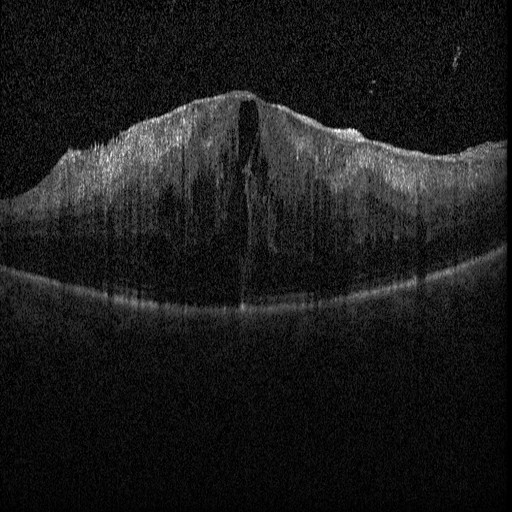 Diagnosis: diabetic macular edema.